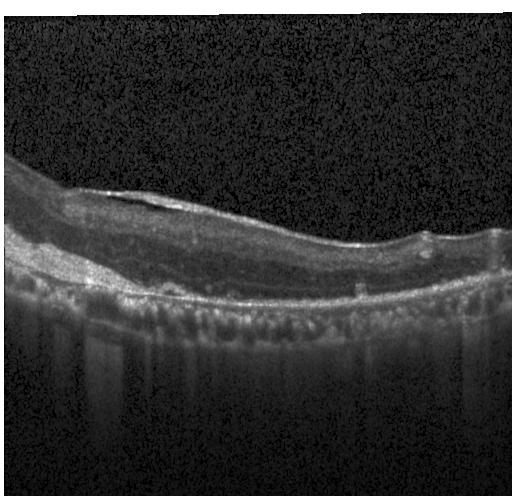 Heidelberg Spectralis · retinal OCT cross-section. Dx: CNV.